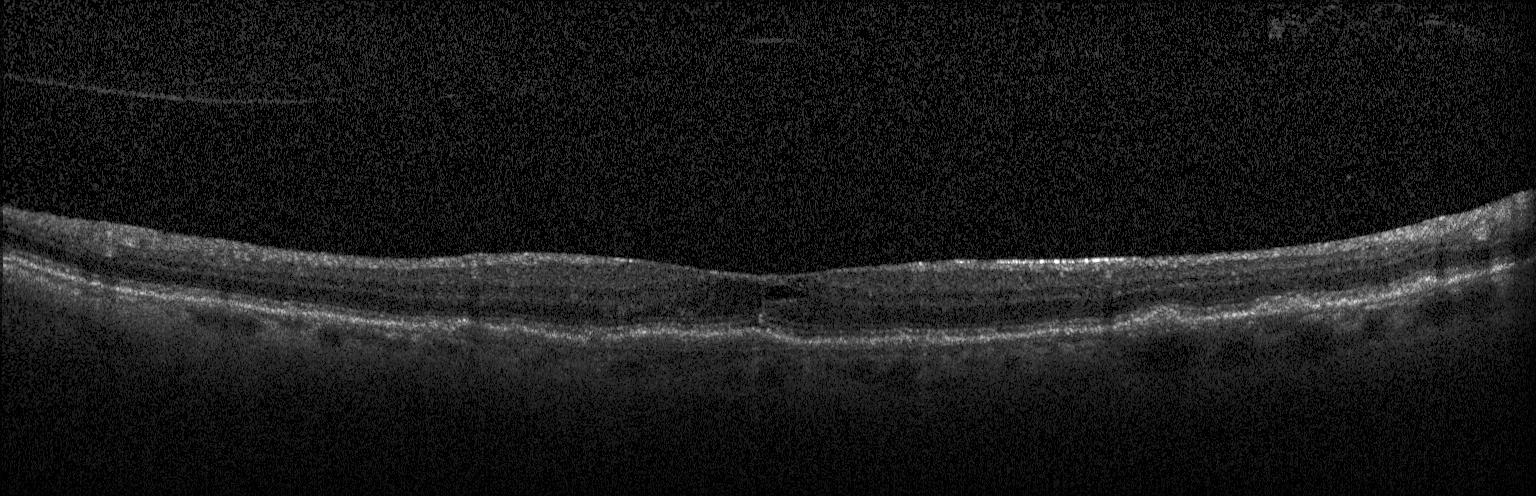 OCT B-scan; instrument: Heidelberg Spectralis.
Assessment: choroidal neovascularization (CNV).